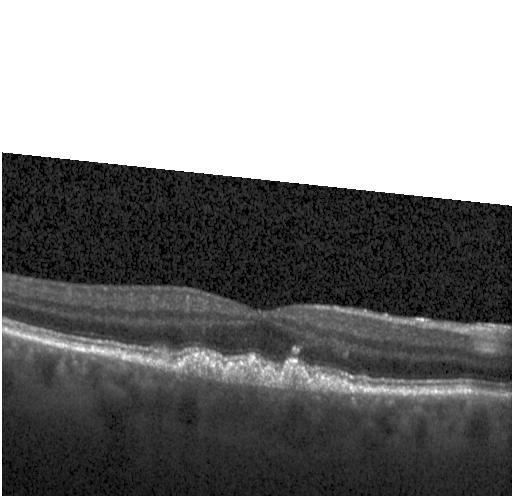 OCT scan showing sub-RPE drusenoid deposits.